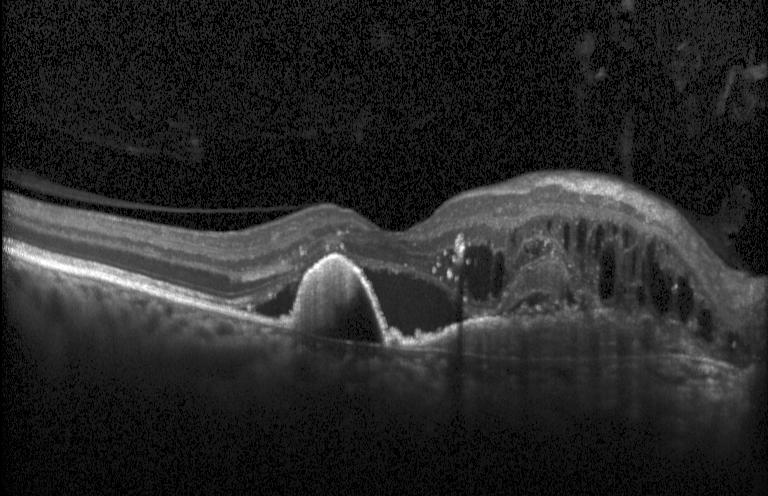

Optical coherence tomography B-scan, macular scan, SD-OCT.
Impression: a choroidal neovascular membrane.